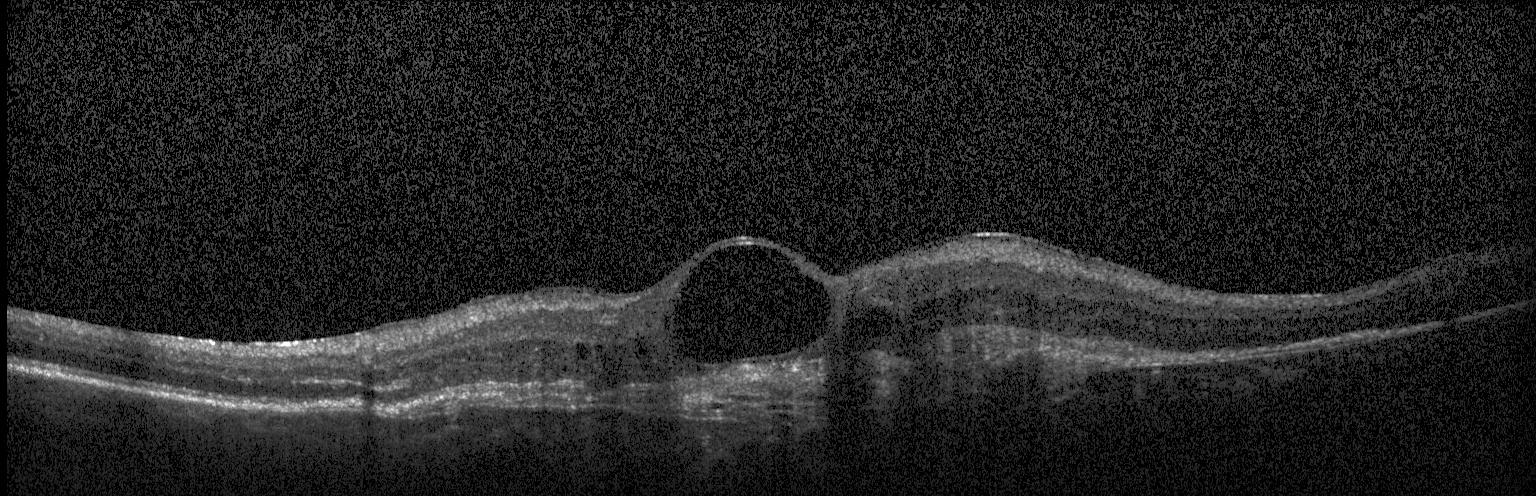

Spectral-domain OCT B-scan: choroidal neovascularization (CNV).